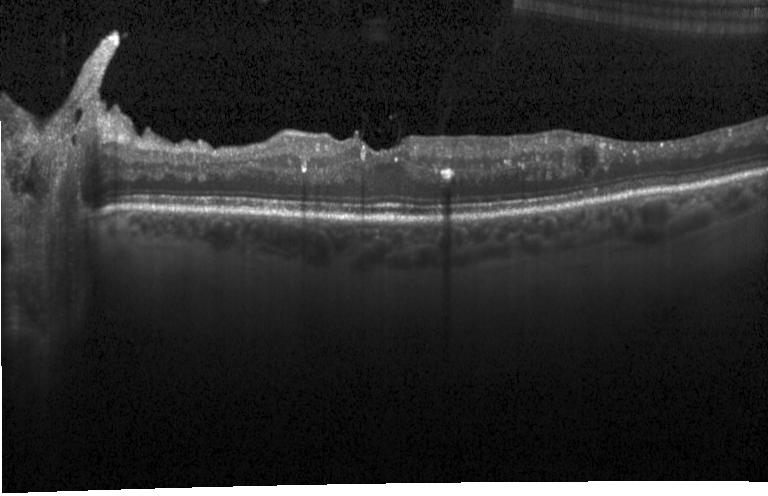 Through the macula · retinal OCT cross-section.
The scan shows DME.